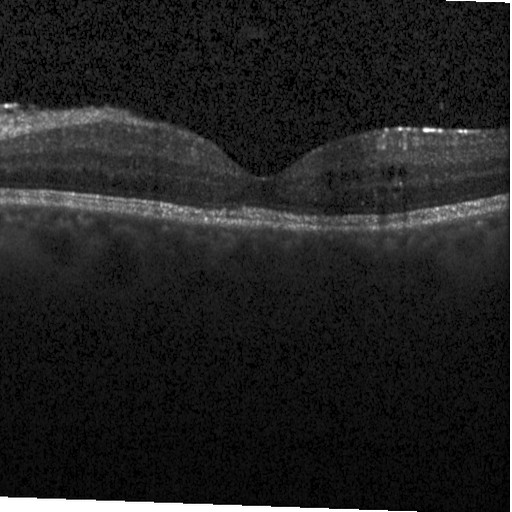
Spectral-domain OCT, optical coherence tomography B-scan.
Diagnosis: DME.